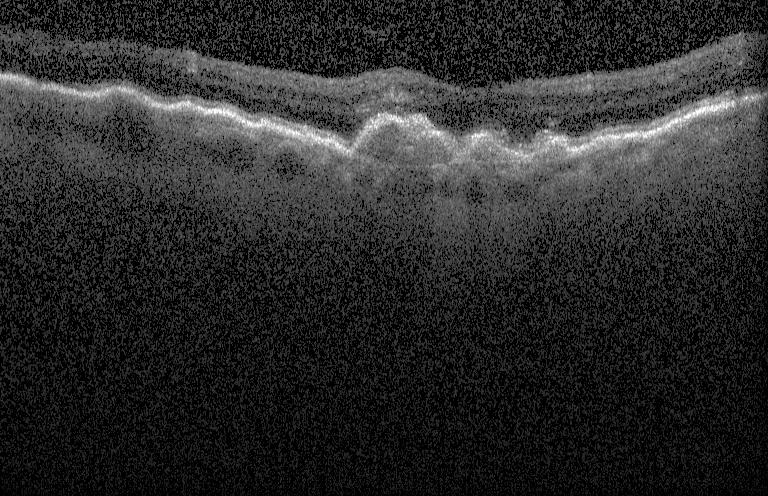 Optical coherence tomography B-scan.
This B-scan demonstrates CNV.